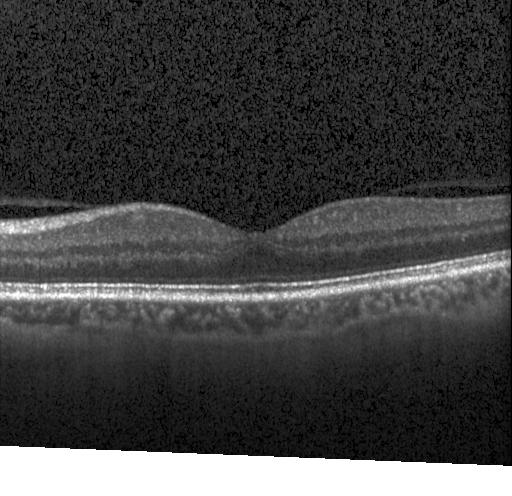
OCT scan showing no choroidal neovascularization, no diabetic macular edema, and no drusen.